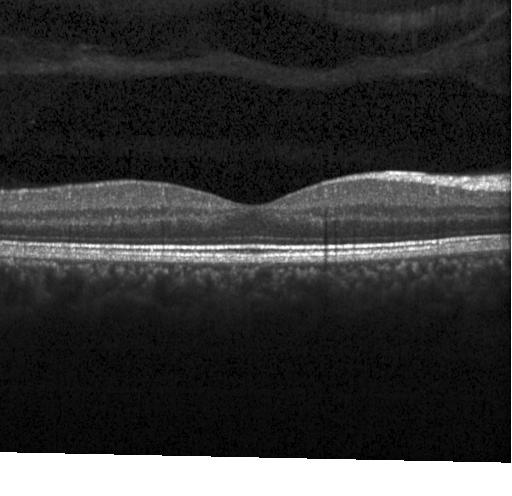

Spectral-domain OCT B-scan: no CNV, no DME, and no drusen.